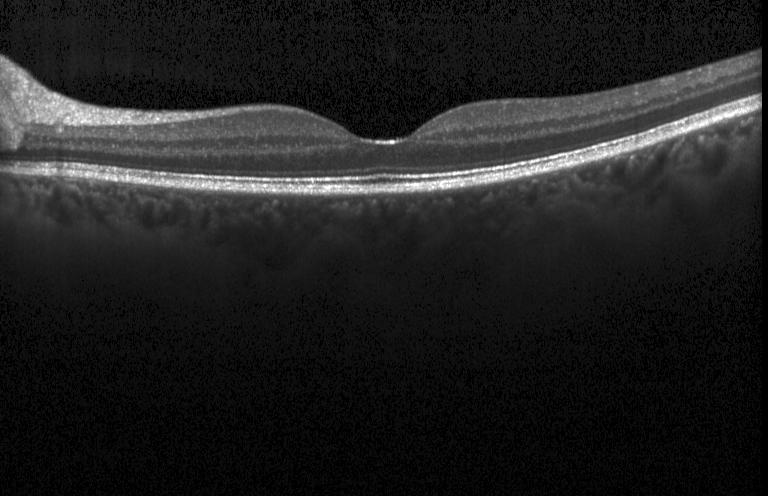
Spectral-domain OCT B-scan: neither choroidal neovascularization, diabetic macular edema, nor drusen.